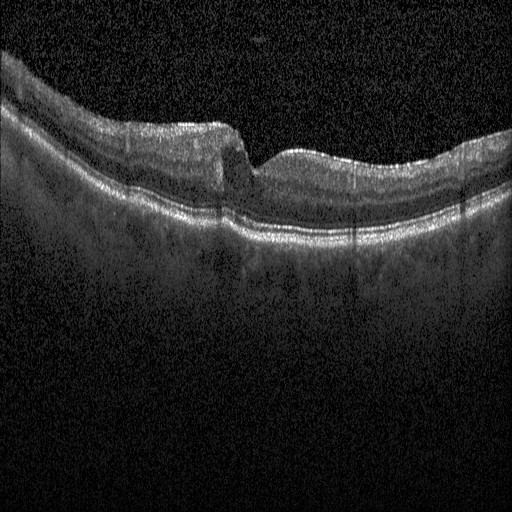 OCT B-scan — The scan shows diabetic macular edema (DME).